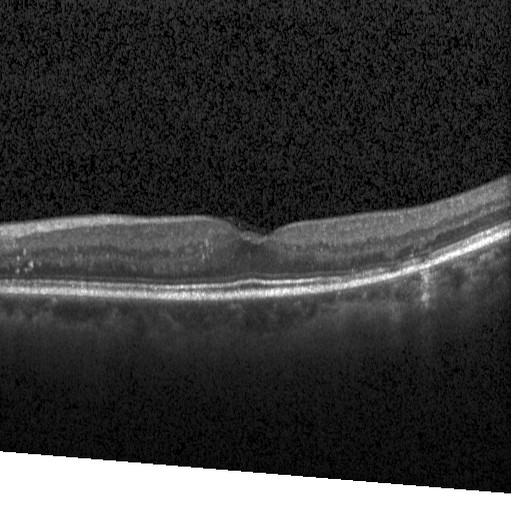

Spectral-domain OCT · fovea-centered · OCT line scan. Dx: diabetic macular edema (DME).